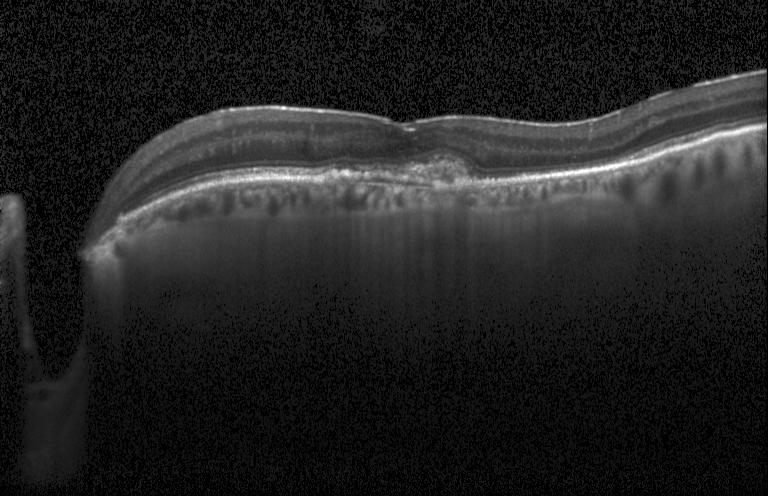 Retinal OCT B-scan. Acquired on a Heidelberg Spectralis. SD-OCT. Macular scan.
This B-scan demonstrates a choroidal neovascular membrane.